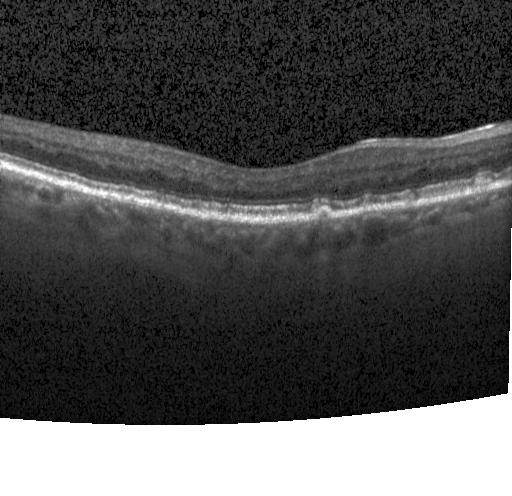

Finding: multiple drusen.